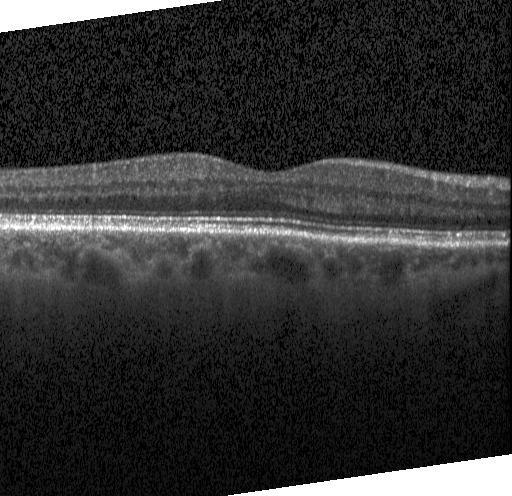
Macular scan · retinal OCT B-scan — Impression: no CNV, no DME, and no drusen.